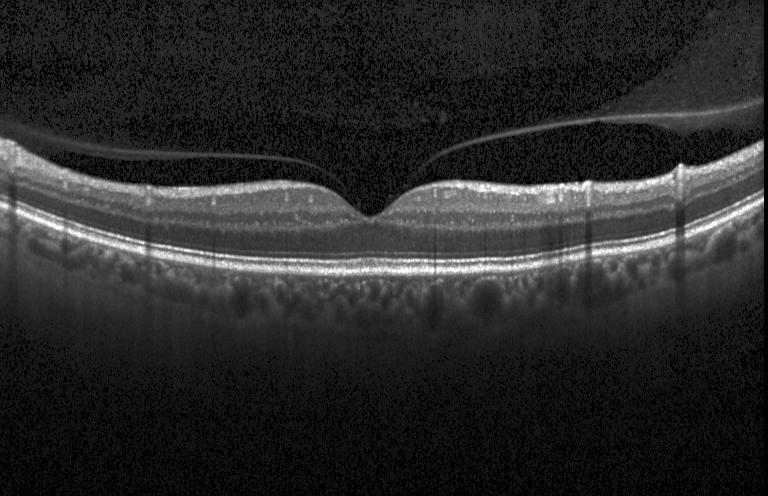

Retinal OCT cross-section.
Diagnosis: no evidence of choroidal neovascularization, diabetic macular edema, or drusen.